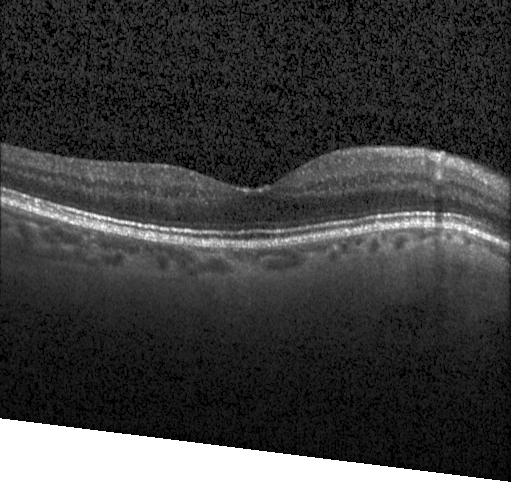 SD-OCT, retinal OCT B-scan — Impression: no choroidal neovascularization, no diabetic macular edema, and no drusen.